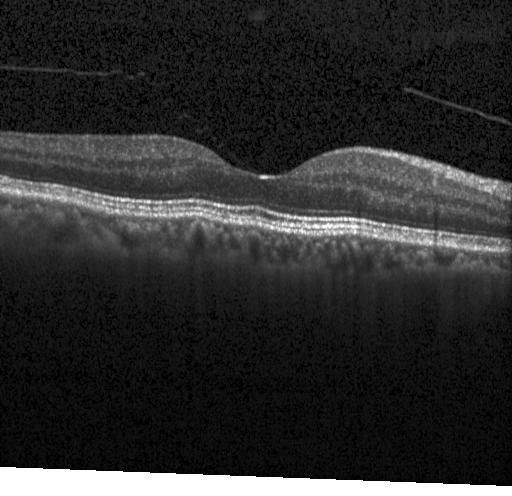 Heidelberg Spectralis; macular scan; OCT line scan. OCT finding: no choroidal neovascularization, diabetic macular edema, or drusen.